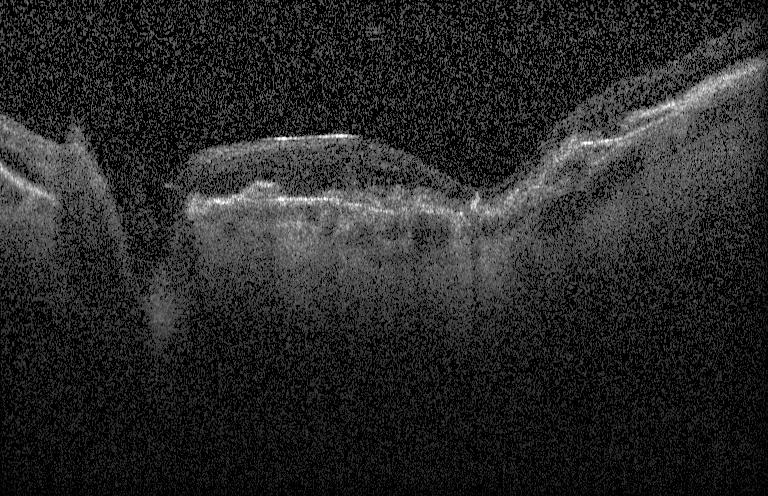

Diagnosis: a choroidal neovascular membrane.